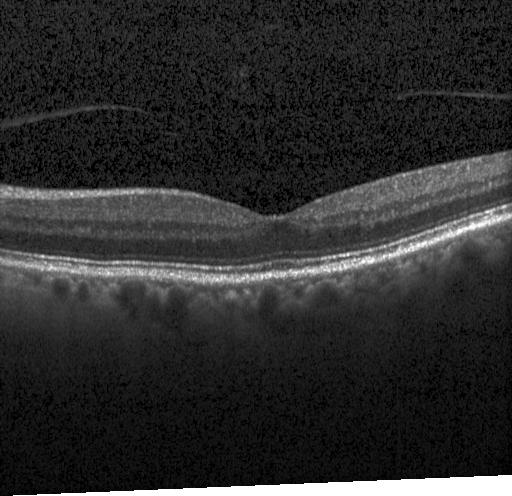

Macular OCT: no evidence of choroidal neovascularization, diabetic macular edema, or drusen.